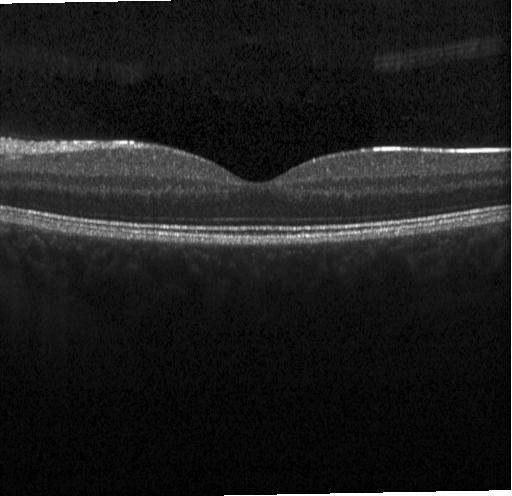
Retinal OCT cross-section; spectral-domain optical coherence tomography; acquired on a Heidelberg Spectralis; fovea-centered.
Dx: neither CNV, DME, nor drusen.